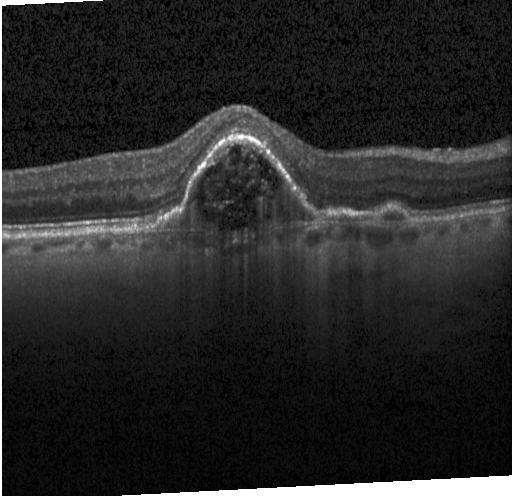

Dx: a choroidal neovascular membrane.